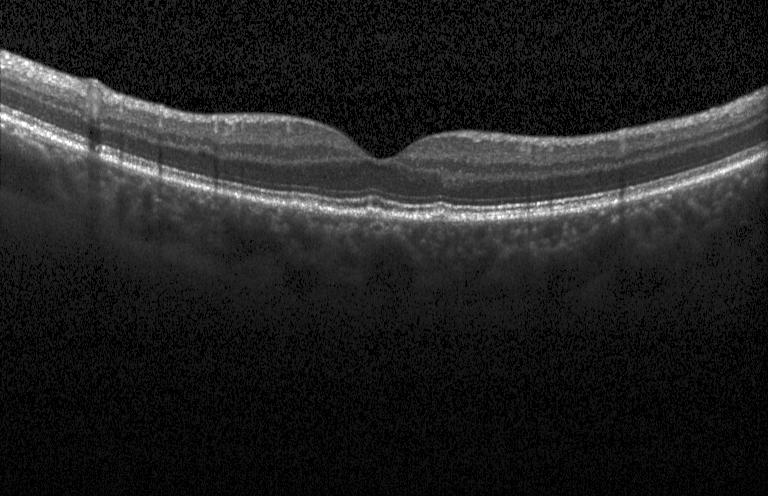 Retinal OCT cross-section showing drusen.